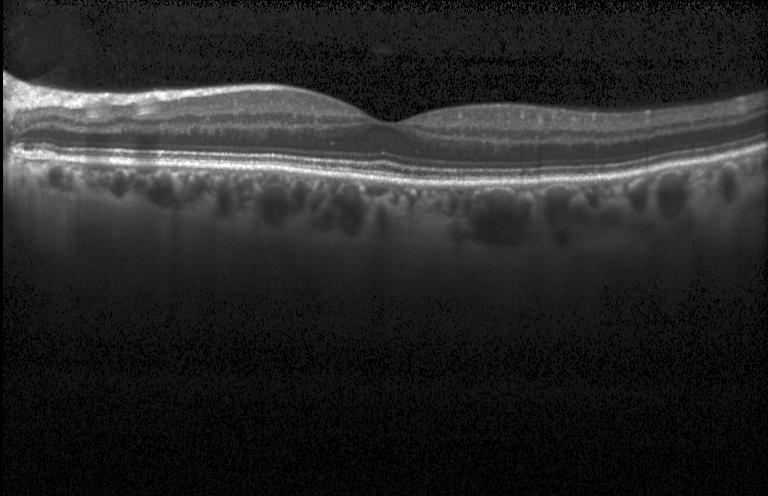

Macular OCT: no choroidal neovascularization, diabetic macular edema, or drusen.